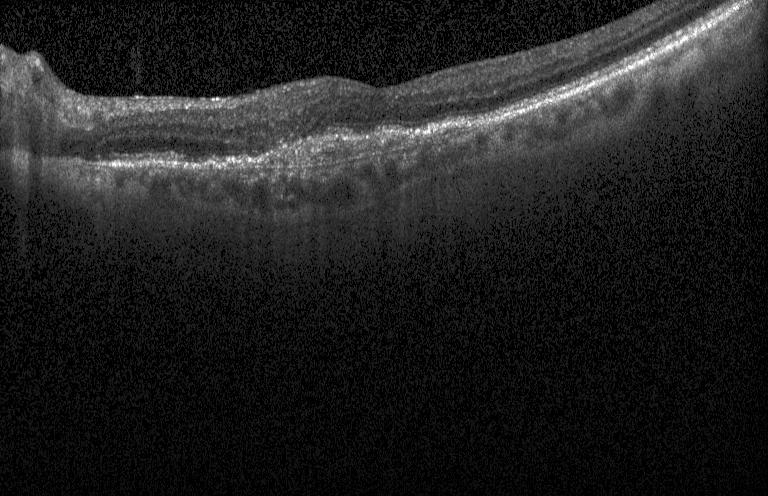 The scan shows CNV.